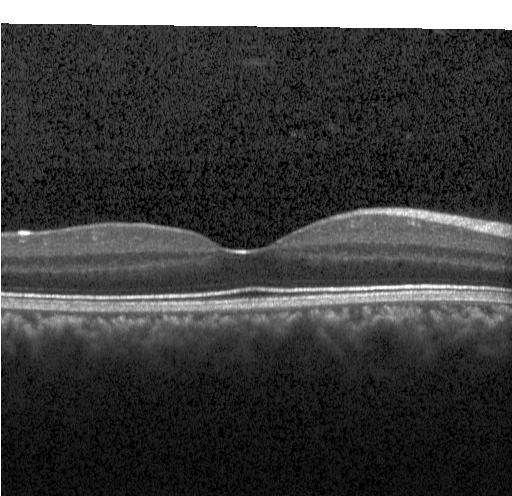
Retinal OCT B-scan, Heidelberg Spectralis, through the macula. No evidence of CNV, DME, or drusen.